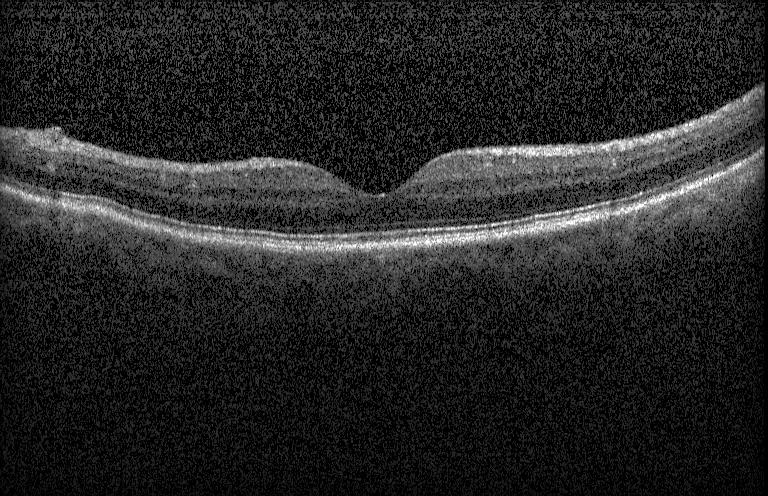 Heidelberg Spectralis · OCT B-scan.
OCT finding: no choroidal neovascularization, no diabetic macular edema, and no drusen.